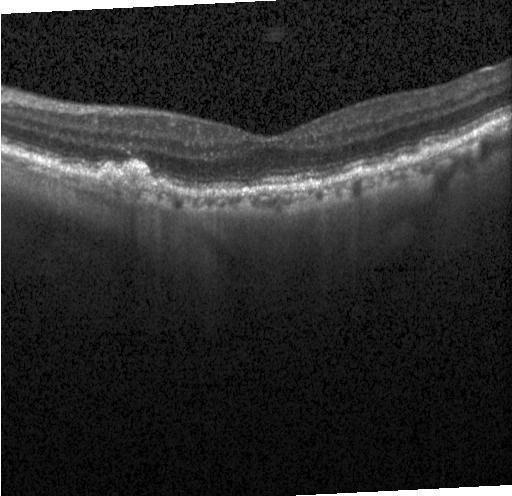
Diagnosis: multiple drusen.